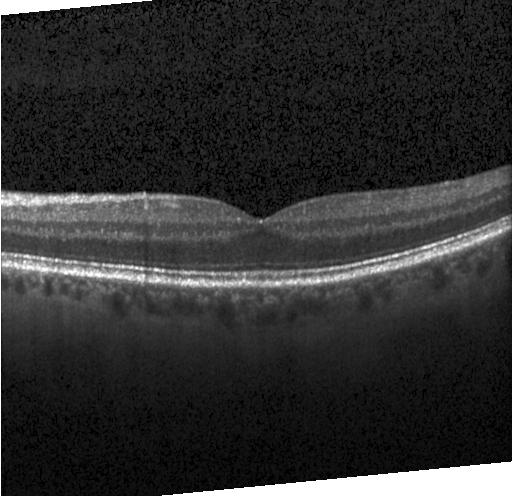
OCT finding: no evidence of CNV, DME, or drusen.